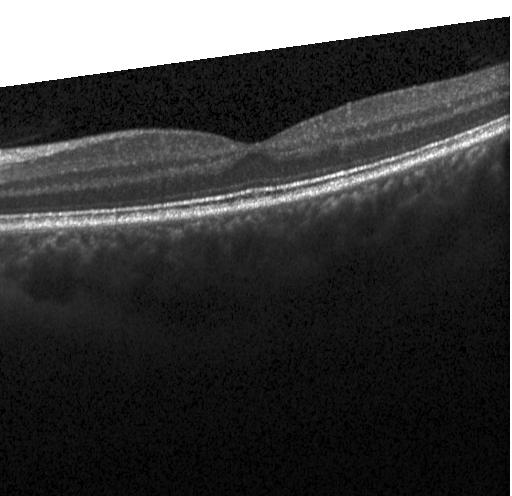

This B-scan demonstrates no CNV, no DME, and no drusen.